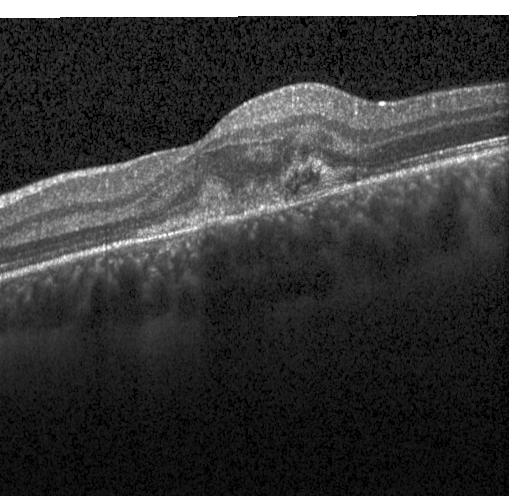
Retinal OCT cross-section. Dx: CNV.